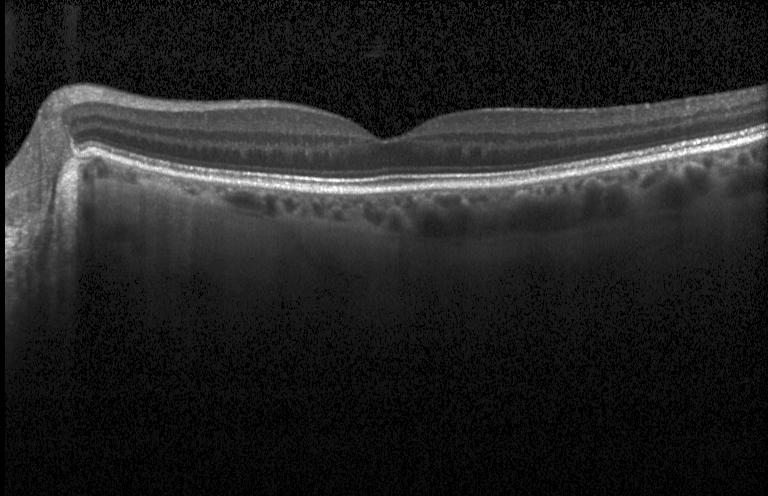 Assessment: no choroidal neovascularization, no diabetic macular edema, and no drusen.